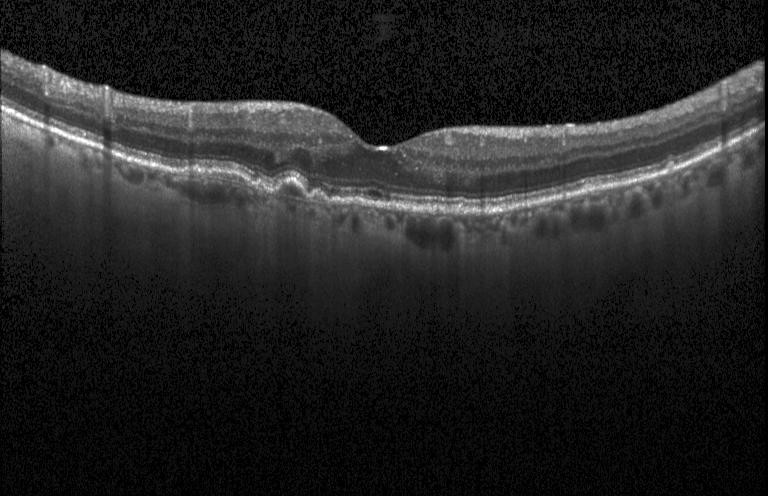

Macular scan · spectral-domain OCT · optical coherence tomography B-scan. OCT finding: drusen.